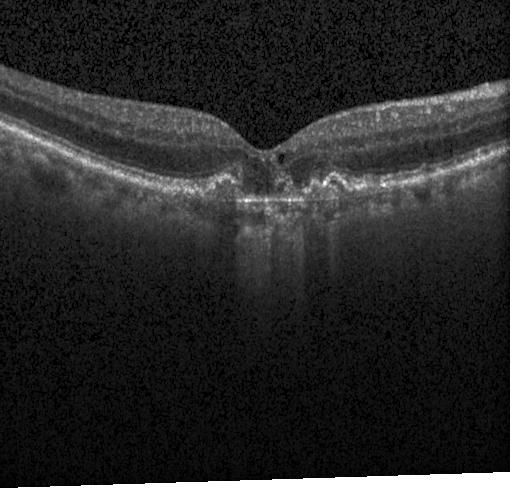

Macular OCT demonstrating a choroidal neovascular membrane.